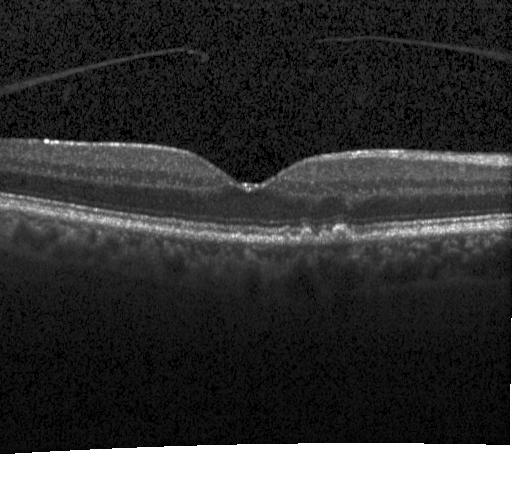 Retinal OCT B-scan — Finding: sub-RPE drusenoid deposits.